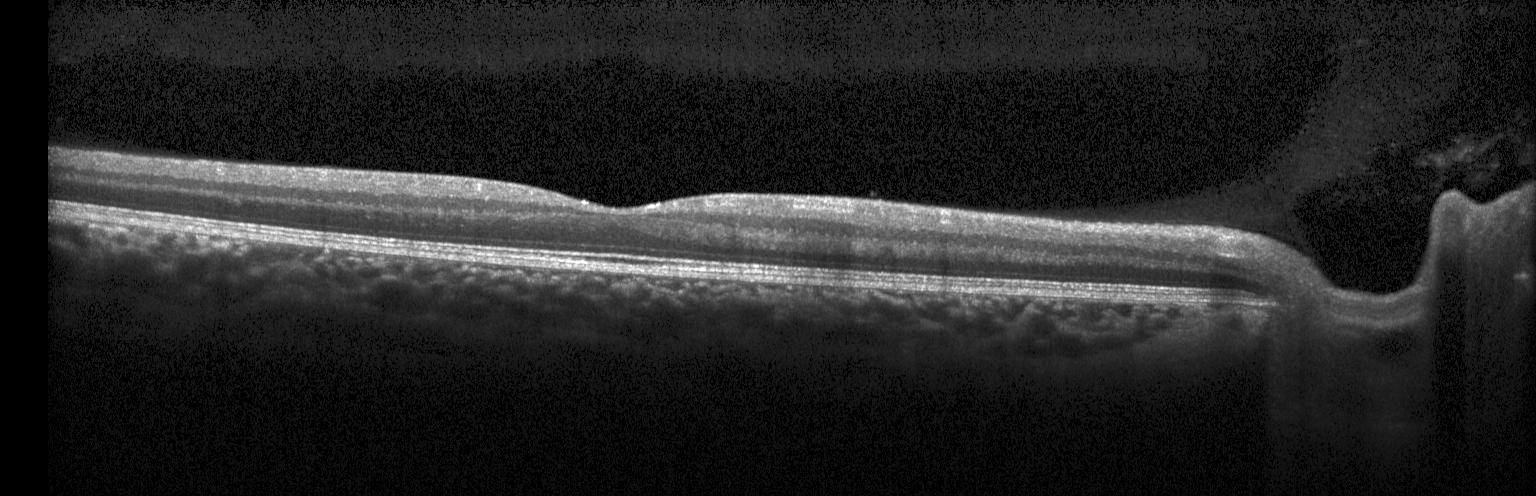 Retinal OCT B-scan. This B-scan demonstrates neither CNV, DME, nor drusen.